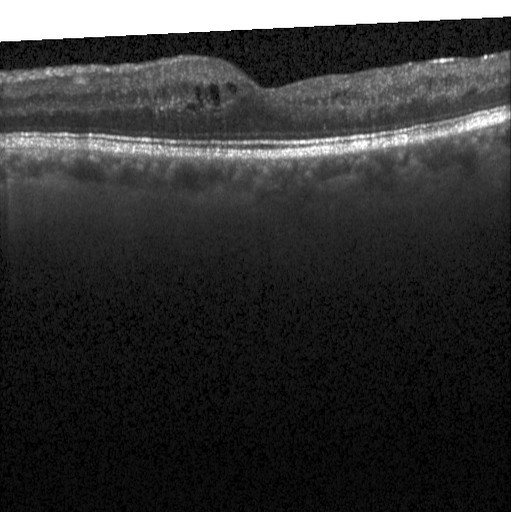

Retinal OCT cross-section; acquired on a Heidelberg Spectralis; horizontal scan through the fovea; spectral-domain OCT.
Impression: DME.